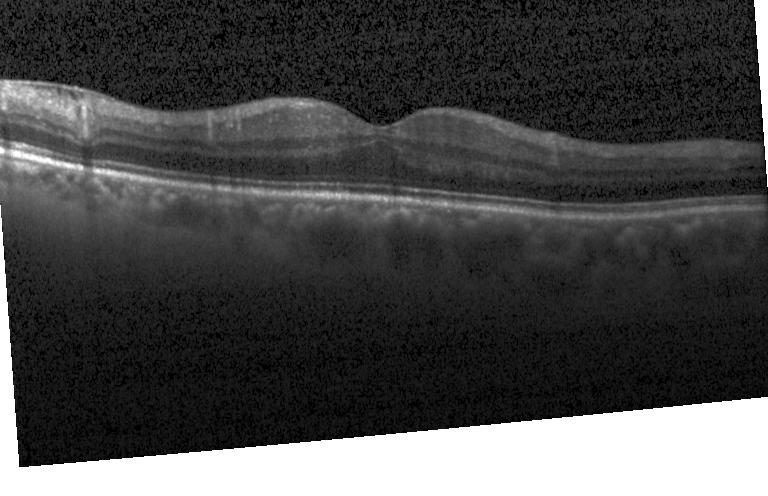

Diagnosis: neither choroidal neovascularization, diabetic macular edema, nor drusen.